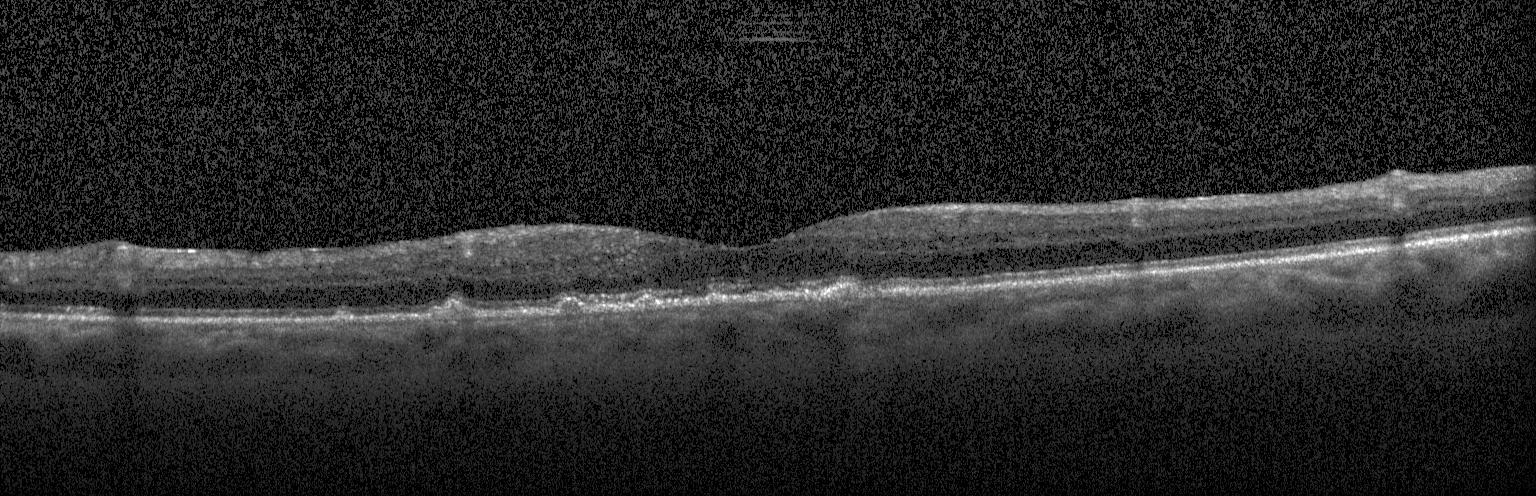

Finding: sub-RPE drusenoid deposits.